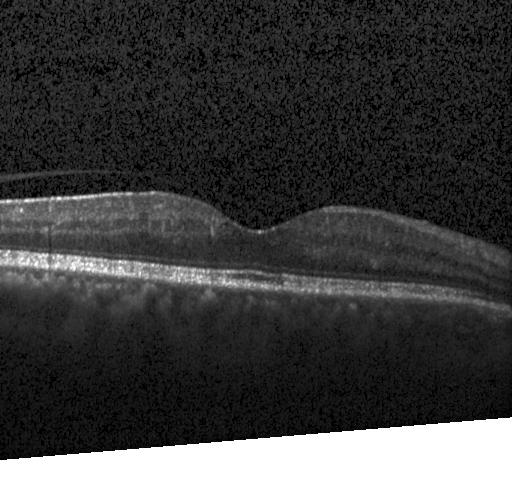

Horizontal scan through the fovea. Heidelberg Spectralis OCT system. Spectral-domain OCT. Retinal OCT B-scan — Macular OCT: neither choroidal neovascularization, diabetic macular edema, nor drusen.